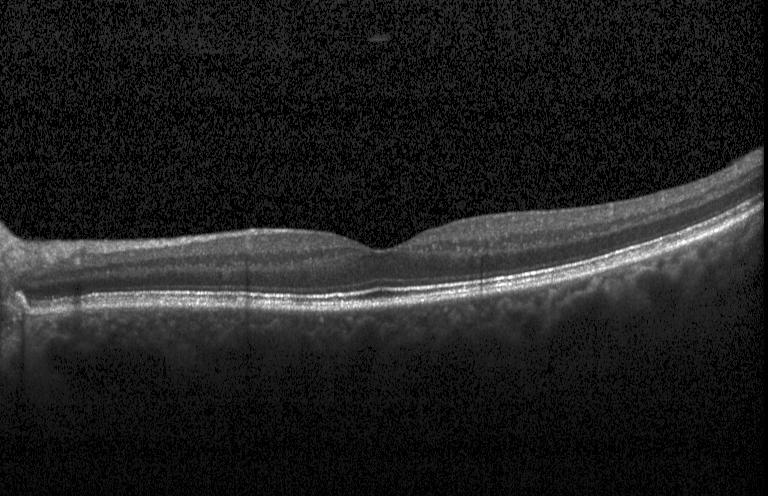
OCT B-scan.
Finding: no evidence of CNV, DME, or drusen.